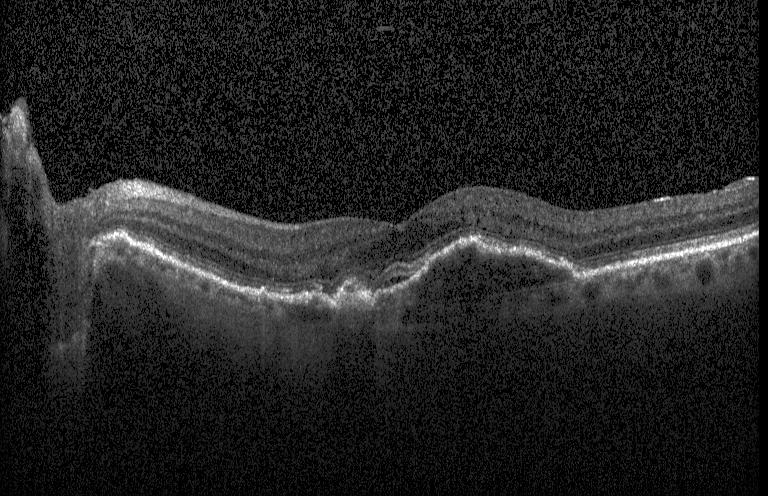
Spectral-domain OCT B-scan: choroidal neovascularization (CNV).